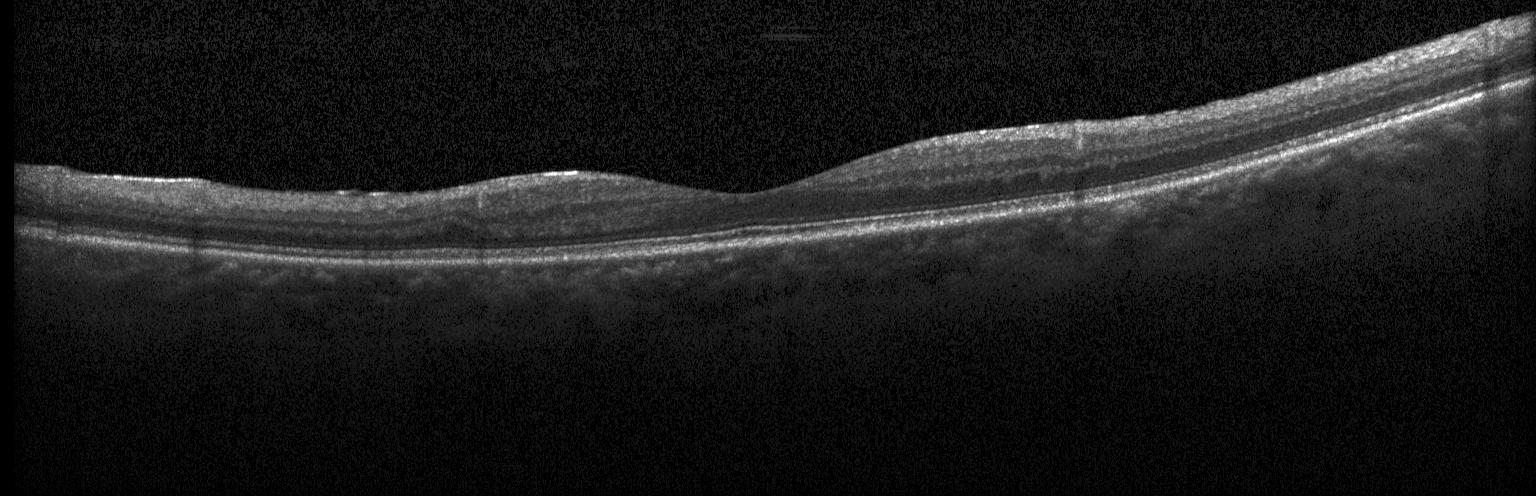 Acquired on a Heidelberg Spectralis. Retinal OCT B-scan. The scan shows no CNV, no DME, and no drusen.